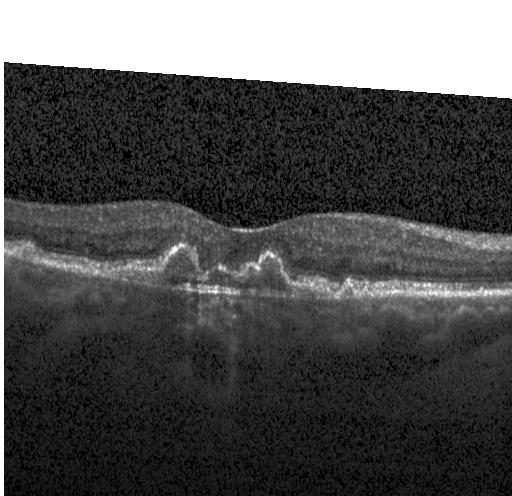

Centered on the fovea, retinal OCT cross-section, SD-OCT. Dx: a choroidal neovascular membrane.